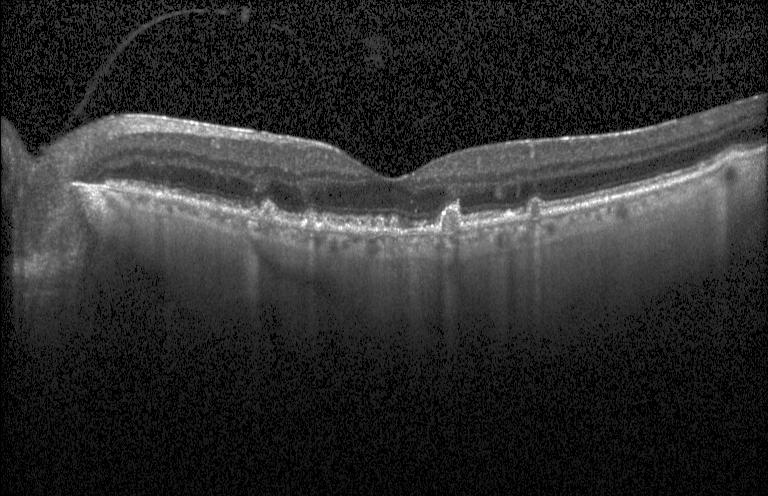
Impression: sub-RPE drusenoid deposits.